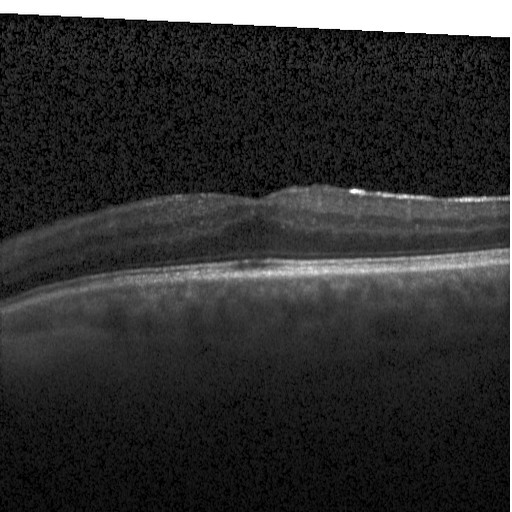 Finding: diabetic macular edema.